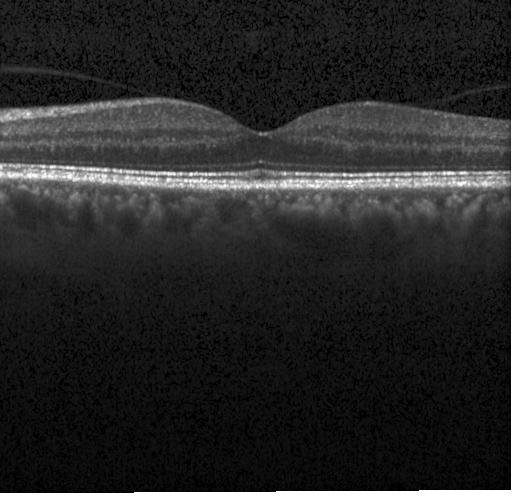
OCT B-scan, spectral-domain optical coherence tomography, Heidelberg Spectralis — Diagnosis: no choroidal neovascularization, diabetic macular edema, or drusen.